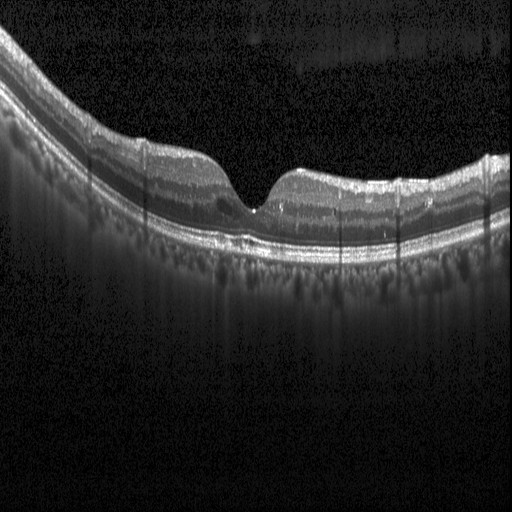

Macular OCT demonstrating DME.